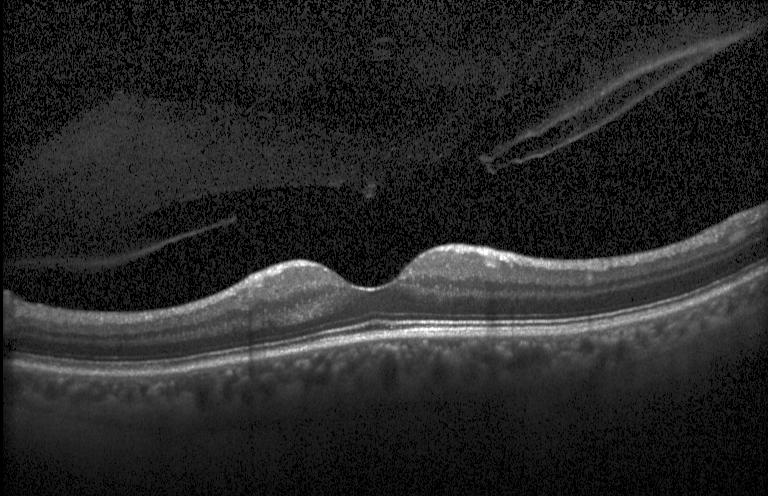
Impression: no CNV, no DME, and no drusen.